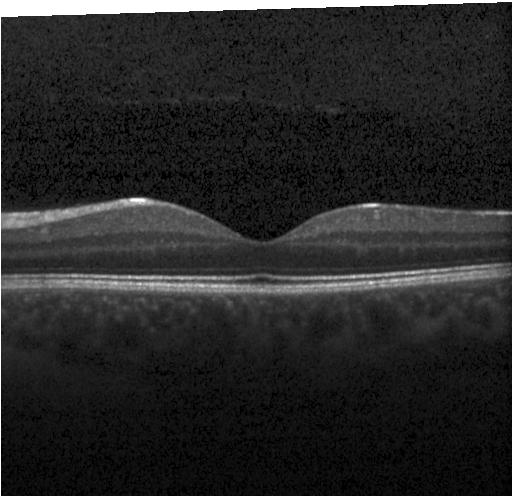 Retinal OCT B-scan, macular scan — Assessment: no evidence of choroidal neovascularization, diabetic macular edema, or drusen.